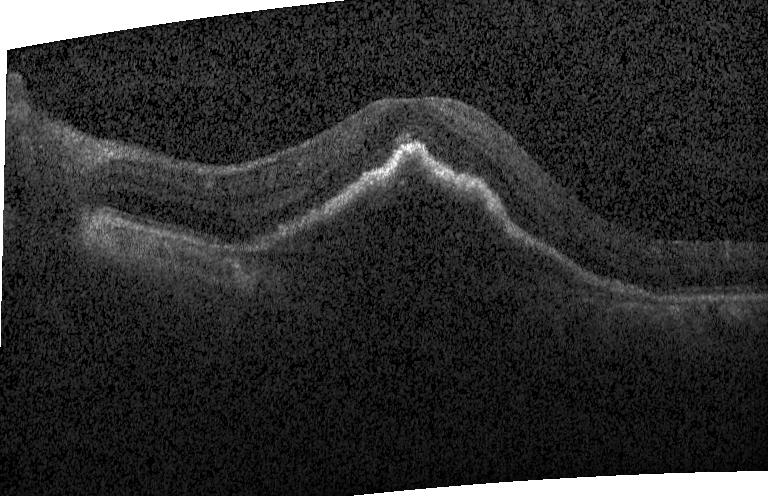 Optical coherence tomography B-scan — Impression: choroidal neovascularization (CNV).